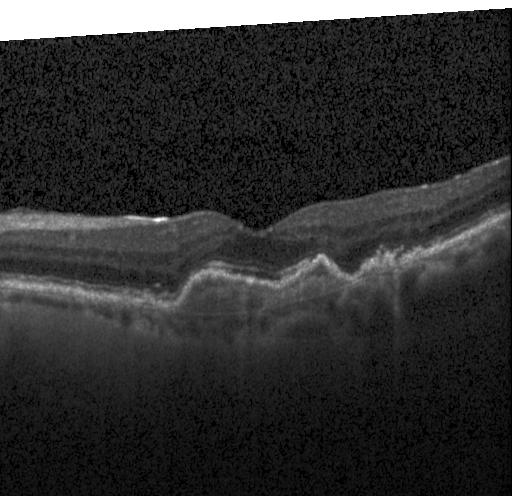

OCT line scan. Heidelberg Spectralis. SD-OCT. Horizontal scan through the fovea. CNV.